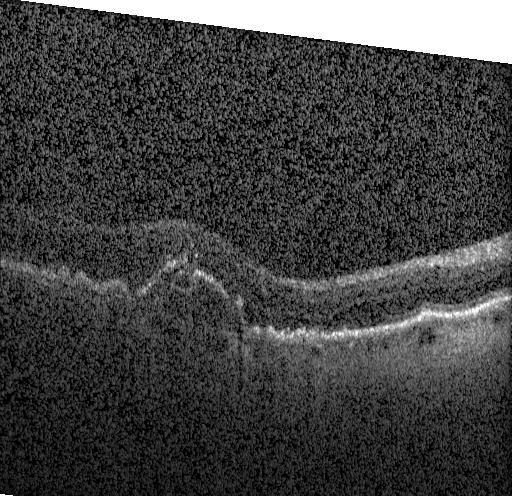 Acquired on a Heidelberg Spectralis, through the macula, spectral-domain OCT, retinal OCT B-scan
Impression: a choroidal neovascular membrane.